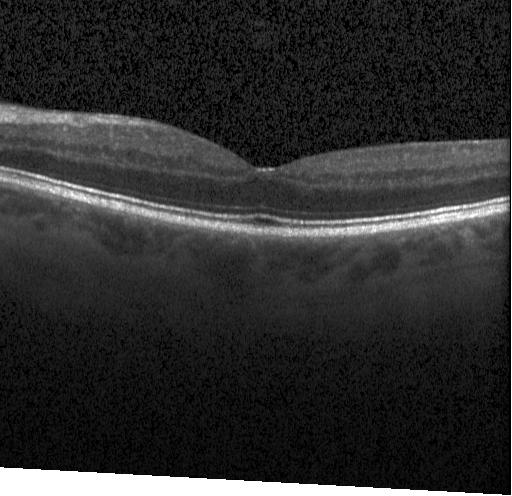
Retinal OCT cross-section. Spectral-domain optical coherence tomography. Horizontal scan through the fovea.
Impression: neither choroidal neovascularization, diabetic macular edema, nor drusen.